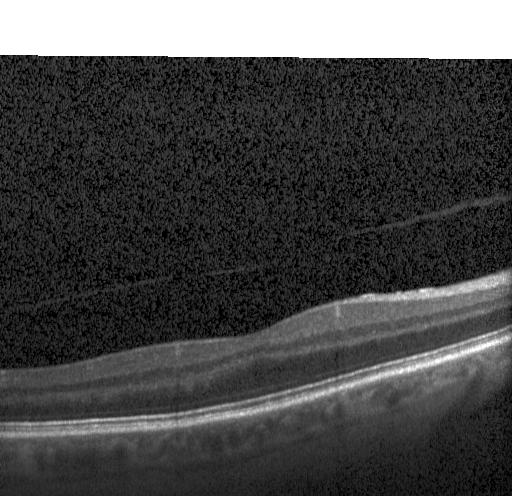 Spectral-domain OCT · centered on the fovea · optical coherence tomography scan · acquired on a Heidelberg Spectralis. The scan shows neither choroidal neovascularization, diabetic macular edema, nor drusen.